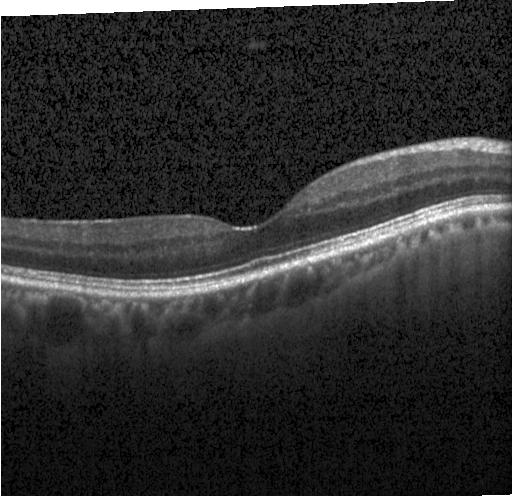
Fovea-centered; optical coherence tomography B-scan — OCT finding: no CNV, no DME, and no drusen.